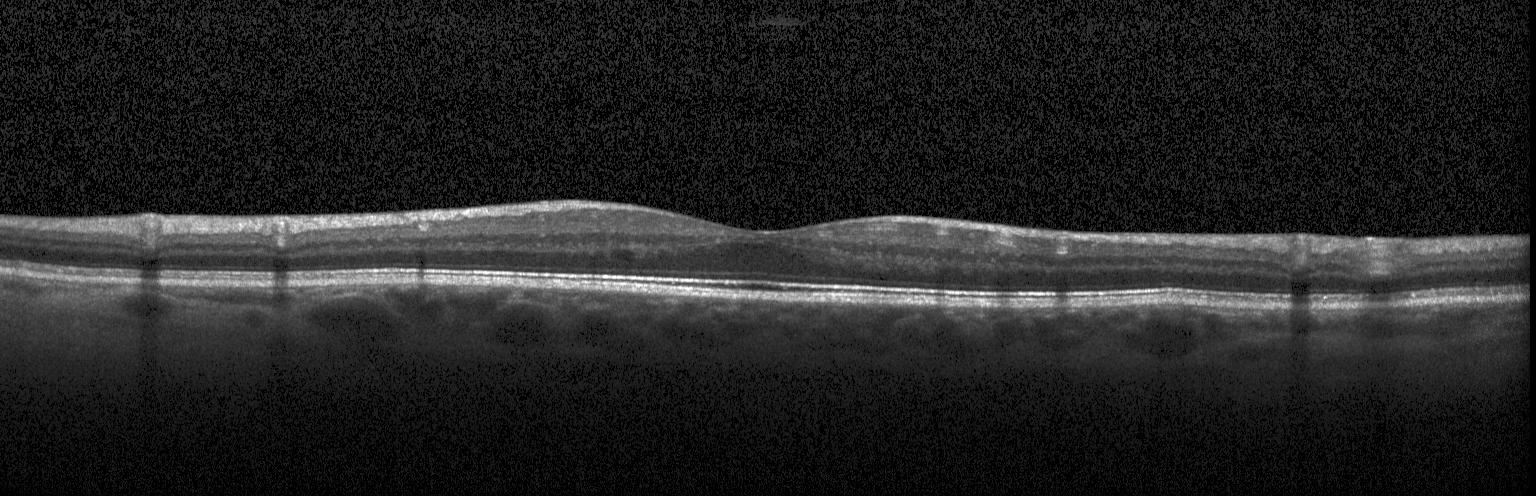 Retinal OCT cross-section showing no evidence of choroidal neovascularization, diabetic macular edema, or drusen.